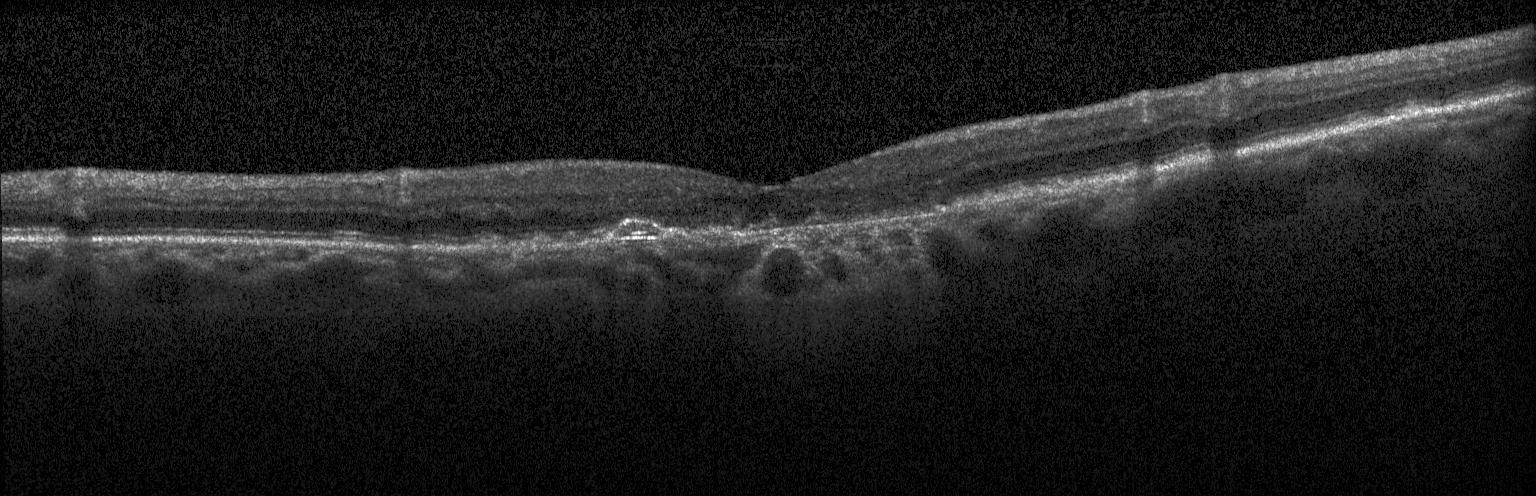

SD-OCT. Horizontal scan through the fovea. Heidelberg Spectralis OCT system. OCT B-scan. CNV.